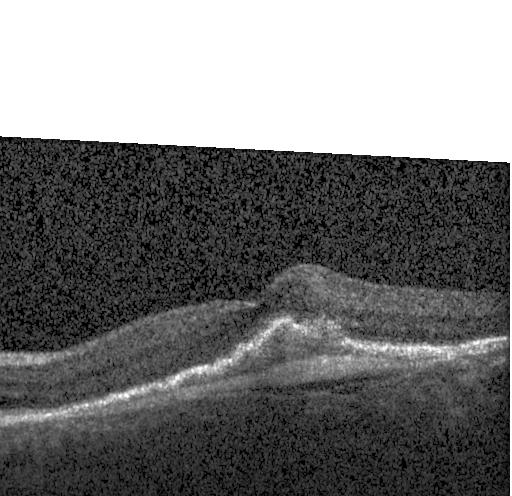
Heidelberg Spectralis OCT system, spectral-domain OCT, OCT B-scan
Finding: a choroidal neovascular membrane.